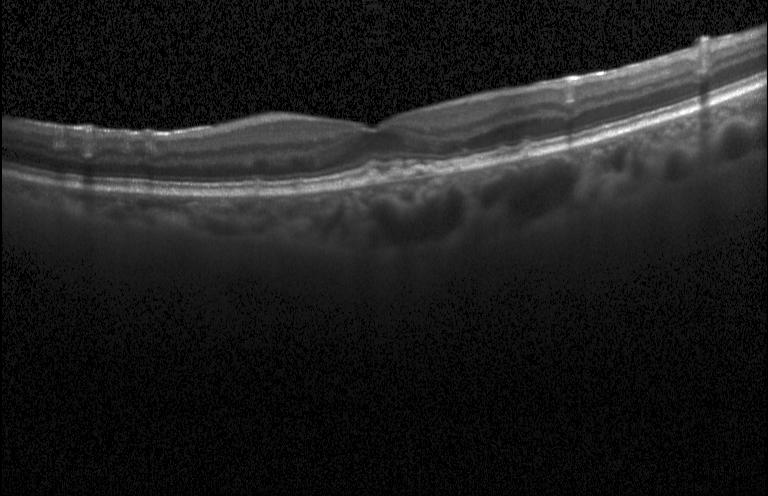 OCT finding: multiple drusen.